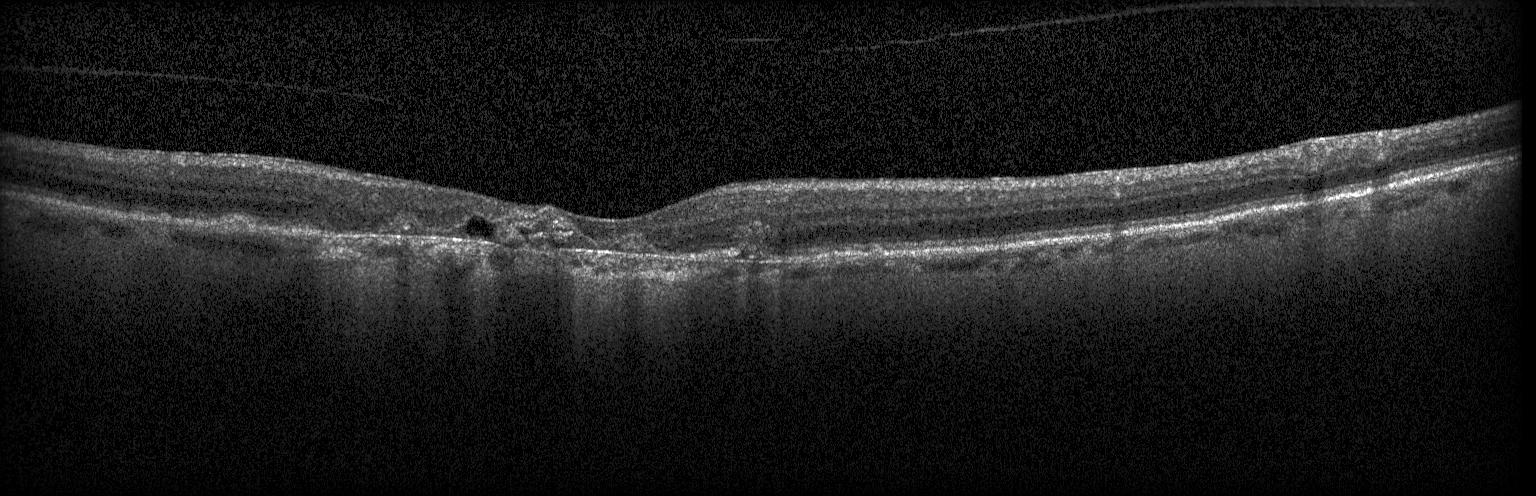

Heidelberg Spectralis. Optical coherence tomography scan. Macular scan. SD-OCT
Assessment: CNV.